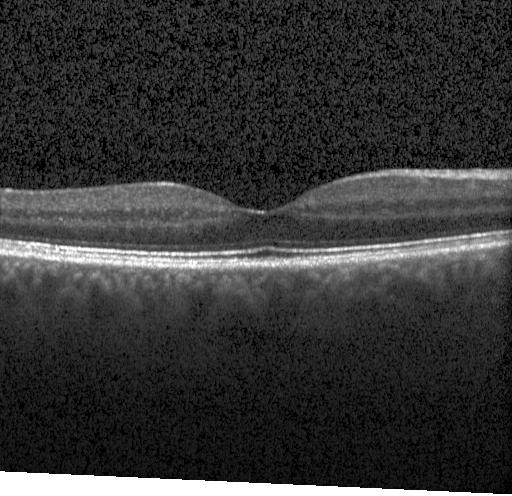

Spectral-domain OCT, acquired on a Heidelberg Spectralis, retinal OCT cross-section
This B-scan demonstrates no CNV, DME, or drusen.